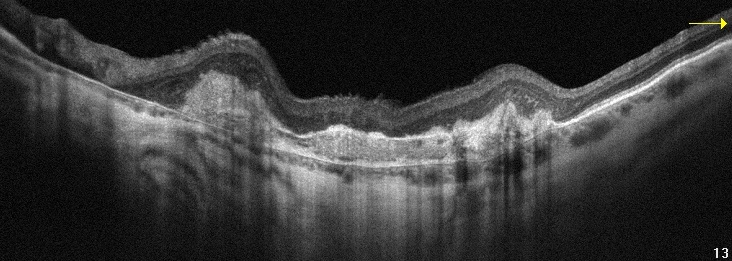

OCT line scan
Finding: age-related macular degeneration.